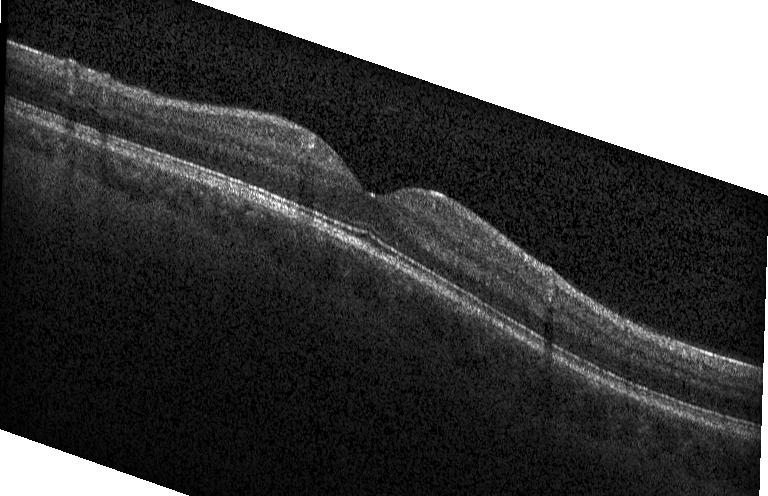

Heidelberg Spectralis · retinal OCT cross-section.
Dx: no evidence of choroidal neovascularization, diabetic macular edema, or drusen.